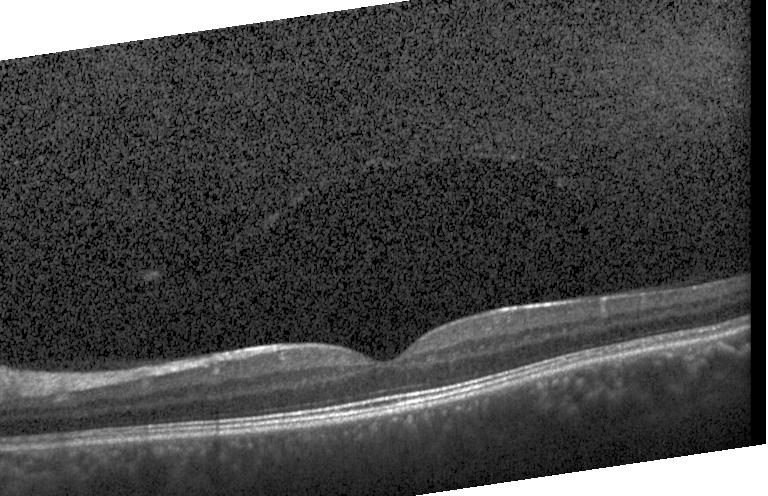

Fovea-centered. Spectral-domain optical coherence tomography. Acquired on a Heidelberg Spectralis. Retinal OCT B-scan
Finding: neither choroidal neovascularization, diabetic macular edema, nor drusen.